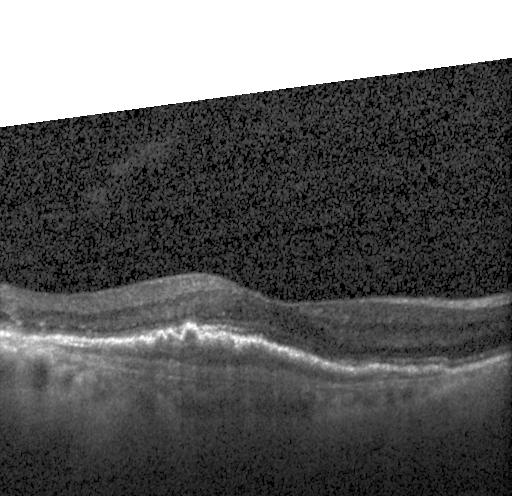

Retinal OCT cross-section showing choroidal neovascularization.